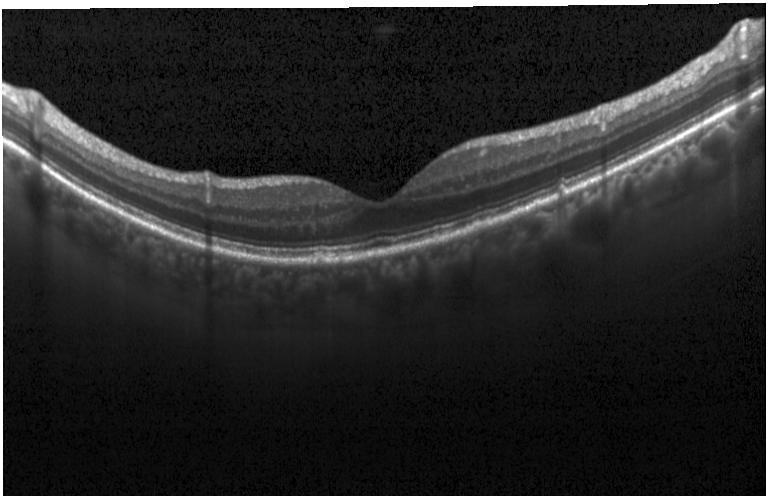 Centered on the fovea, acquired on a Heidelberg Spectralis, retinal OCT B-scan, spectral-domain OCT.
Assessment: no choroidal neovascularization, no diabetic macular edema, and no drusen.